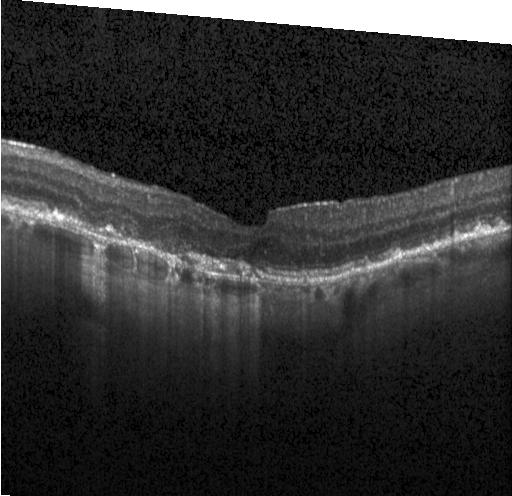
Spectral-domain OCT B-scan: neither choroidal neovascularization, diabetic macular edema, nor drusen.